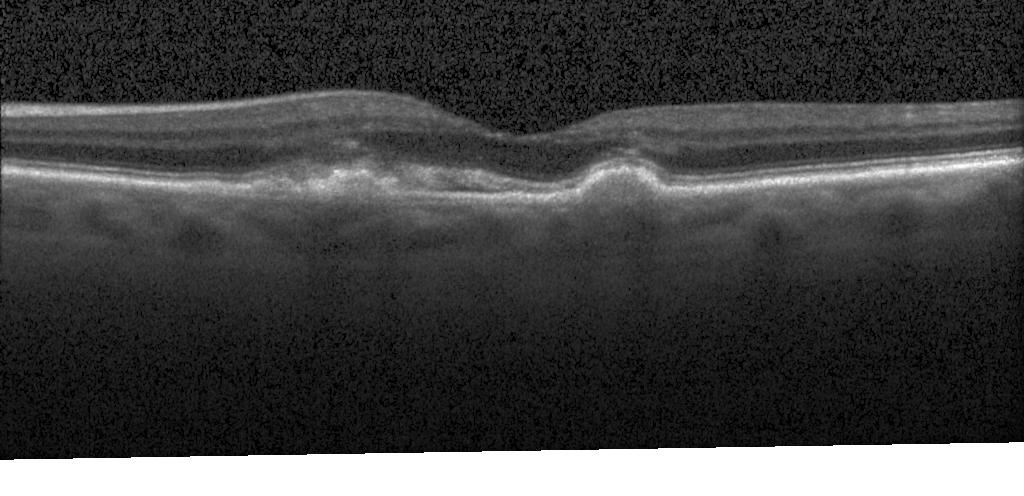
OCT line scan · Heidelberg Spectralis.
This B-scan demonstrates choroidal neovascularization.